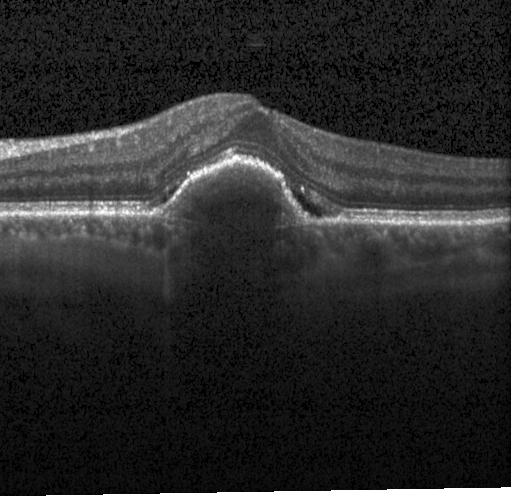

Impression: choroidal neovascularization (CNV).